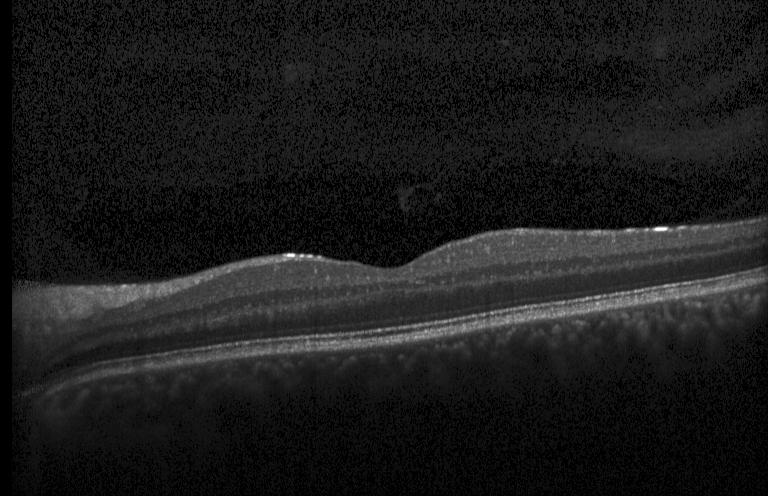
OCT B-scan showing no choroidal neovascularization, no diabetic macular edema, and no drusen.